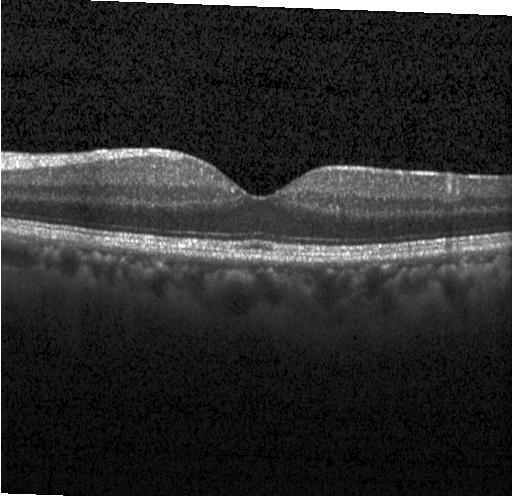 OCT line scan. This B-scan demonstrates no evidence of CNV, DME, or drusen.